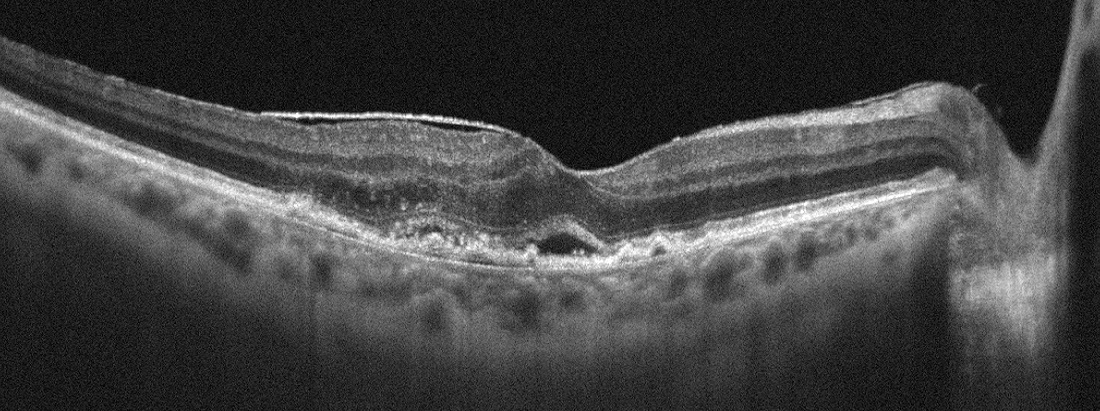
The scan shows AMD.